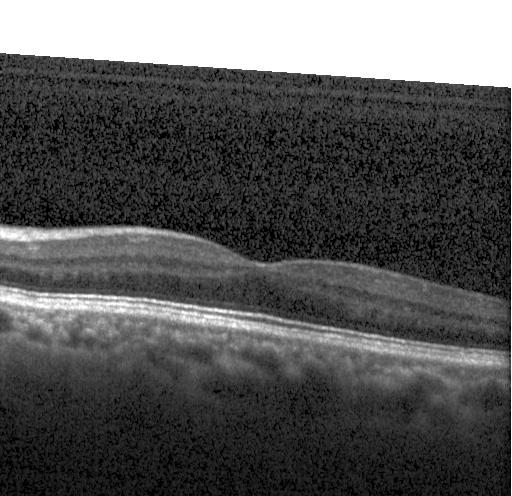
OCT finding: no choroidal neovascularization, no diabetic macular edema, and no drusen.